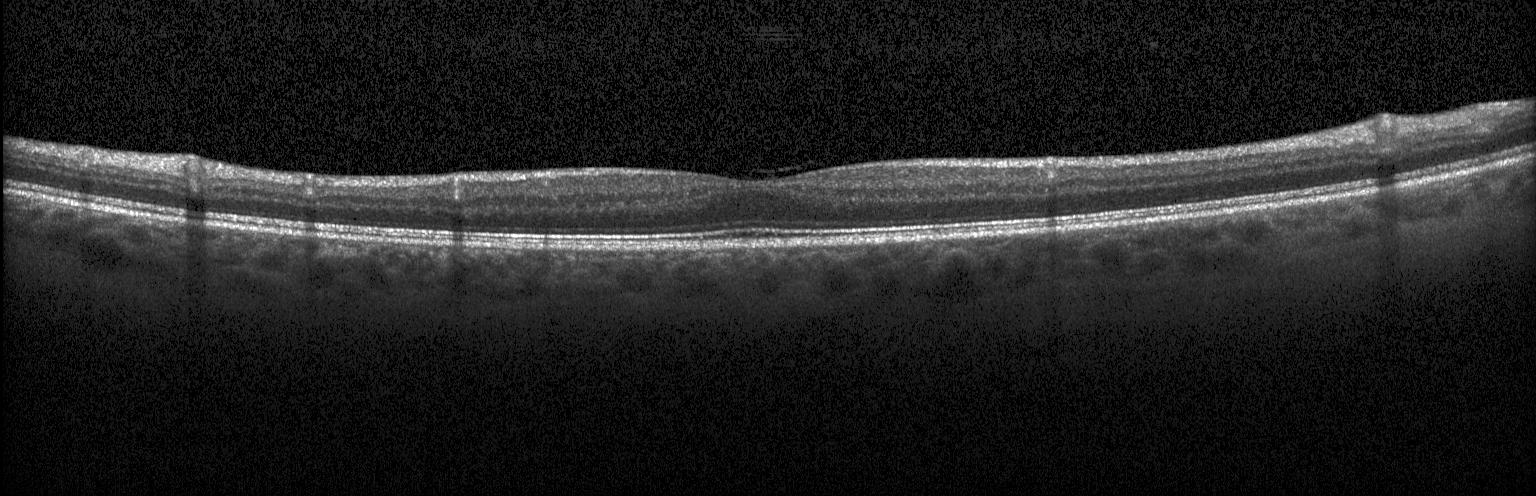
Spectral-domain optical coherence tomography, through the macula, OCT B-scan, acquired on a Heidelberg Spectralis
Finding: no choroidal neovascularization, diabetic macular edema, or drusen.